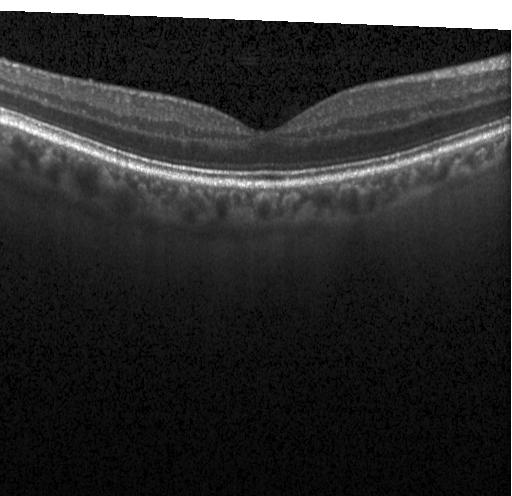 Through the macula; optical coherence tomography B-scan; spectral-domain optical coherence tomography; Heidelberg Spectralis.
Diagnosis: neither CNV, DME, nor drusen.